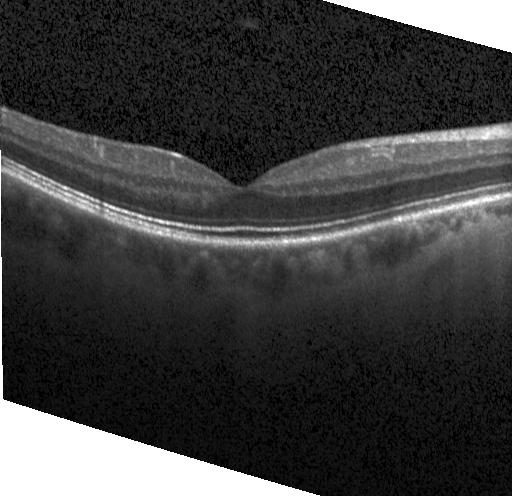 Optical coherence tomography B-scan, Heidelberg Spectralis, centered on the fovea, spectral-domain OCT
Diagnosis: no evidence of choroidal neovascularization, diabetic macular edema, or drusen.